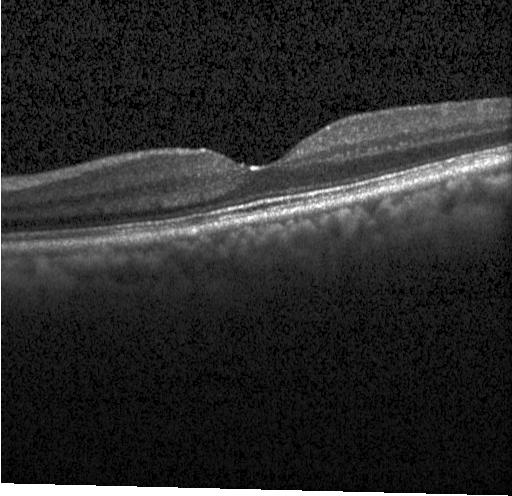

Finding: no choroidal neovascularization, no diabetic macular edema, and no drusen.